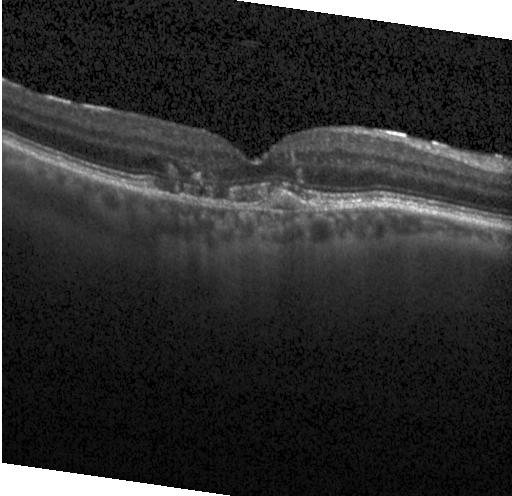 Retinal OCT B-scan — Assessment: choroidal neovascularization (CNV).